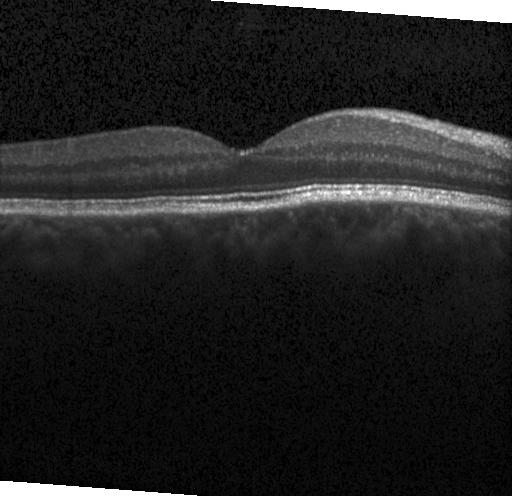
Heidelberg Spectralis, horizontal scan through the fovea, retinal OCT cross-section
OCT finding: neither CNV, DME, nor drusen.